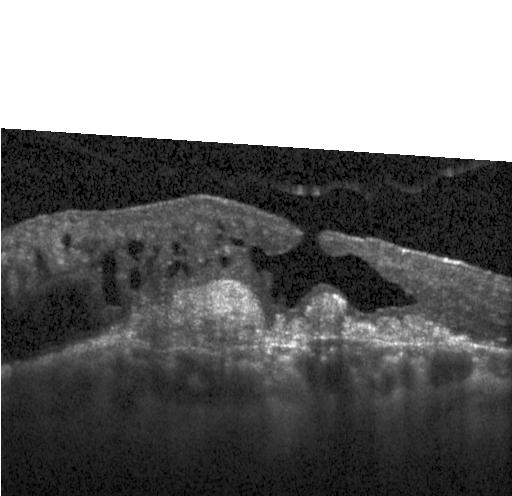 Instrument: Heidelberg Spectralis · spectral-domain optical coherence tomography · retinal OCT B-scan · horizontal scan through the fovea
Impression: a choroidal neovascular membrane.